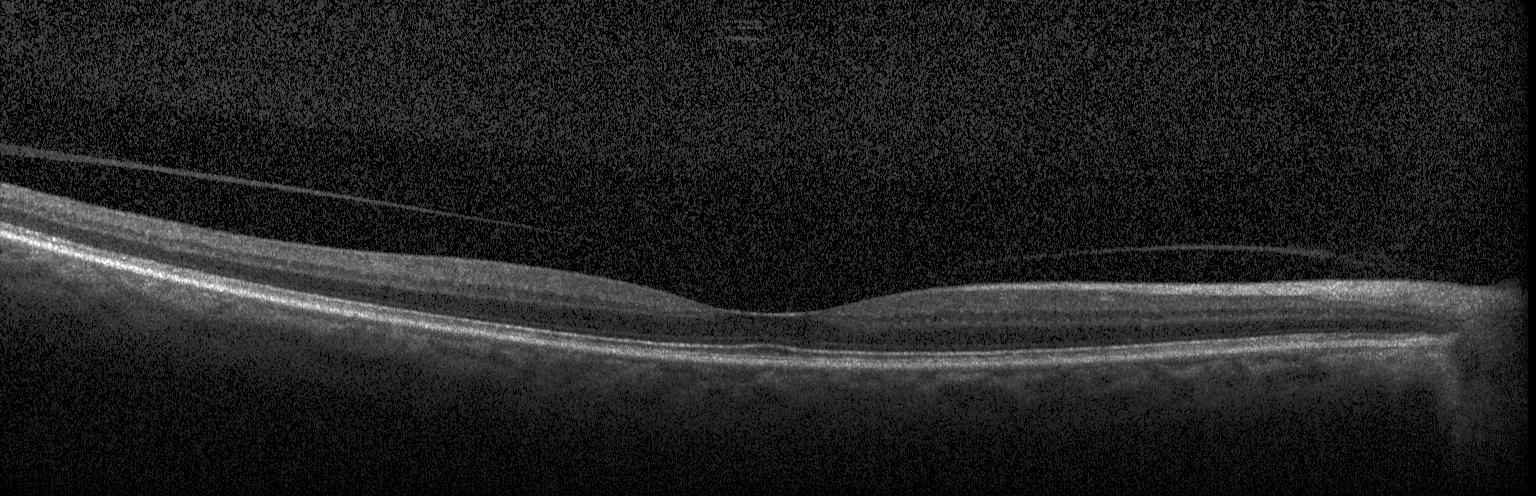
Diagnosis: no choroidal neovascularization, no diabetic macular edema, and no drusen.